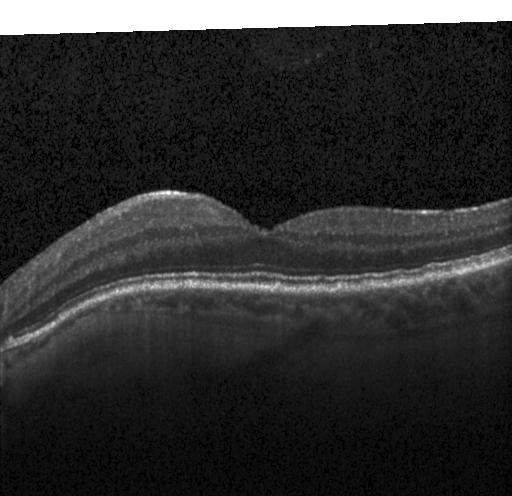

Dx: sub-RPE drusenoid deposits.